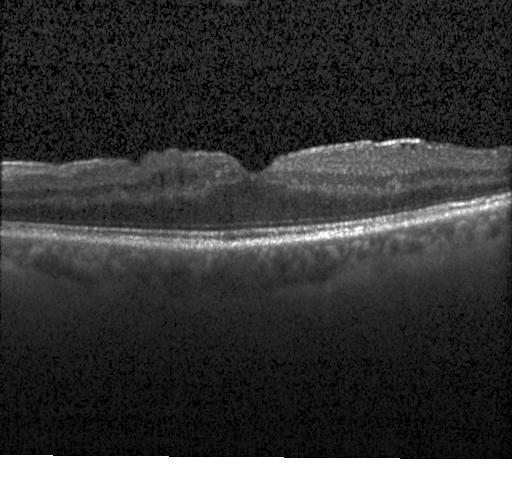

Retinal OCT B-scan.
The scan shows diabetic macular edema.